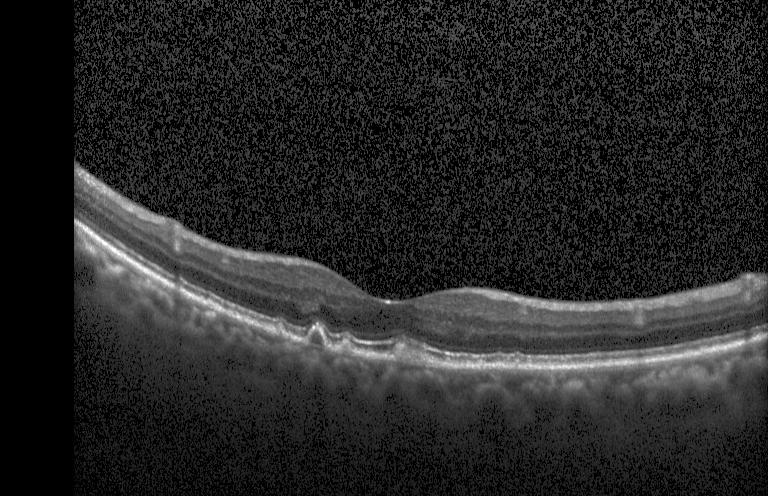 Optical coherence tomography scan · fovea-centered.
Impression: multiple drusen.